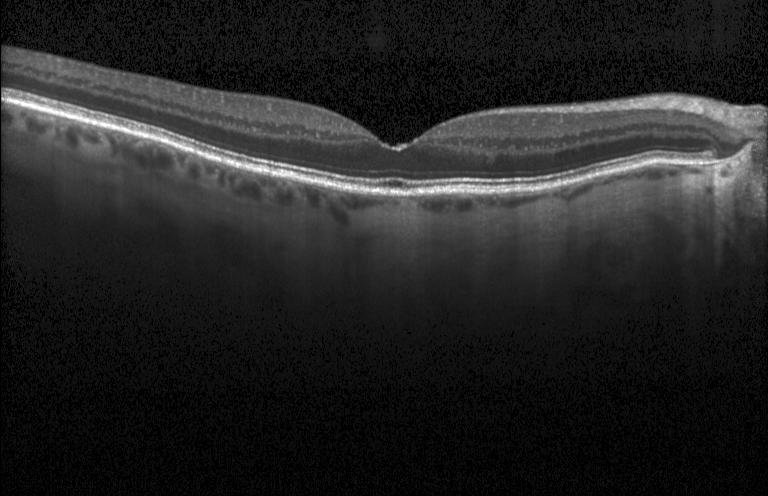
Macular scan, Heidelberg Spectralis OCT system, optical coherence tomography scan. Macular OCT: no choroidal neovascularization, diabetic macular edema, or drusen.